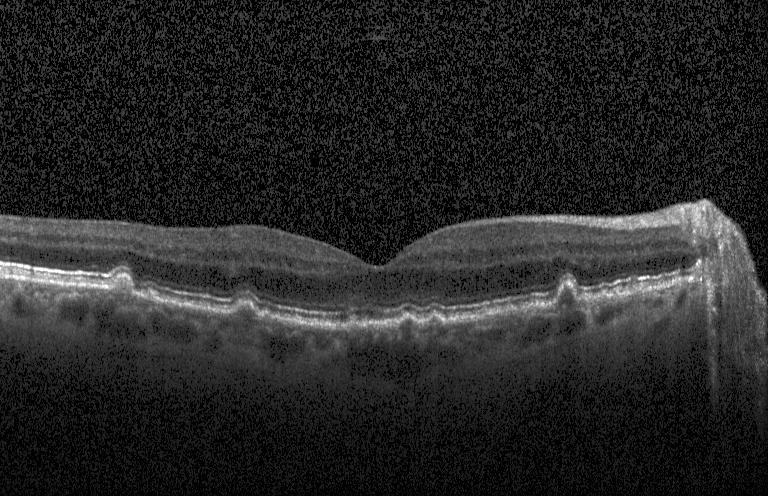
Optical coherence tomography B-scan · spectral-domain optical coherence tomography — This B-scan demonstrates multiple drusen.